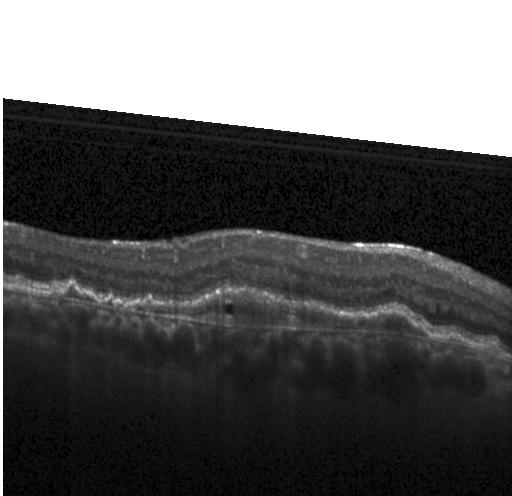

Assessment: CNV.